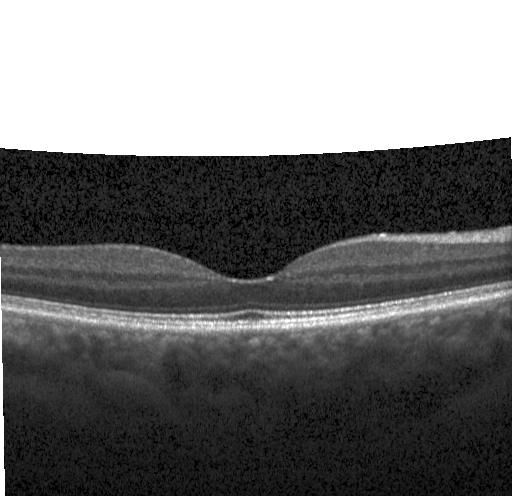
Diagnosis: neither choroidal neovascularization, diabetic macular edema, nor drusen.